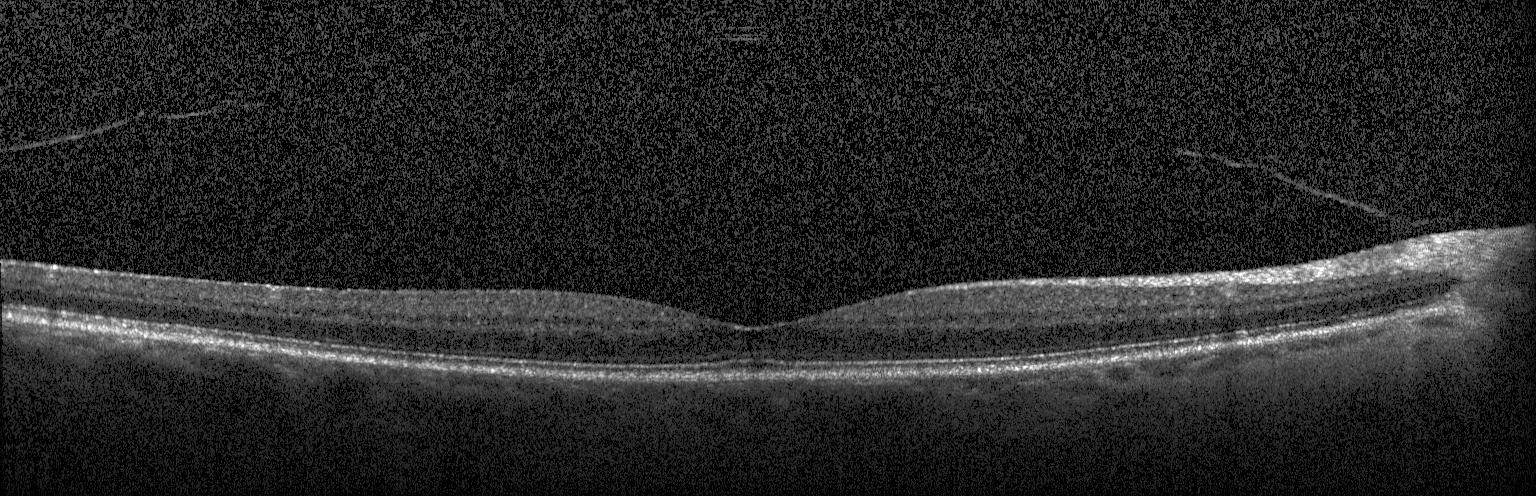

Spectral-domain optical coherence tomography. Optical coherence tomography scan. Heidelberg Spectralis. Through the macula.
This B-scan demonstrates neither choroidal neovascularization, diabetic macular edema, nor drusen.